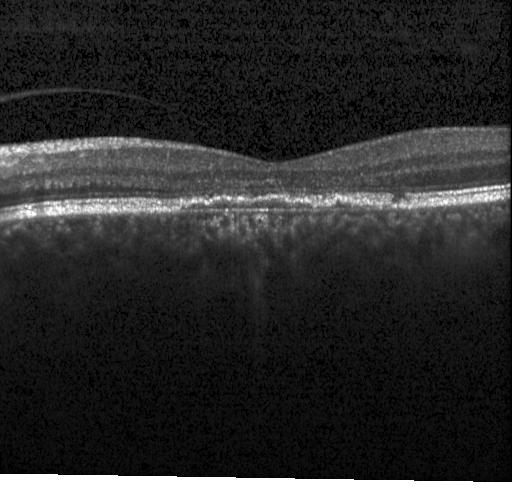

Spectral-domain OCT; centered on the fovea; optical coherence tomography scan. A choroidal neovascular membrane.